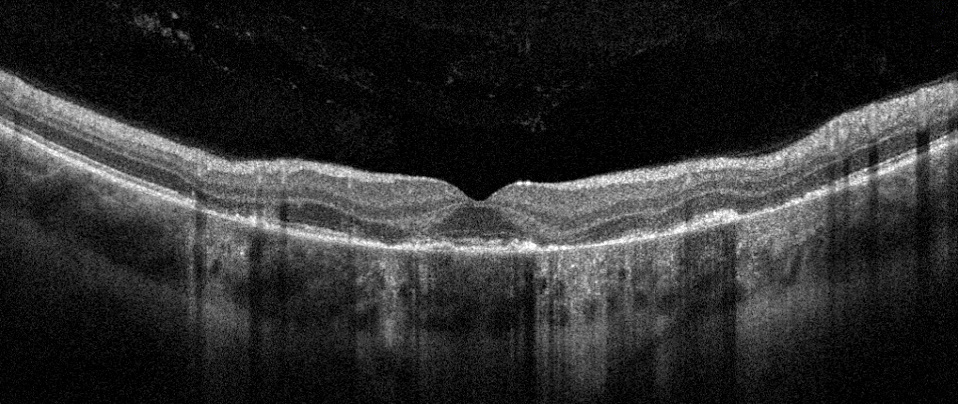
OCT finding: age-related macular degeneration.